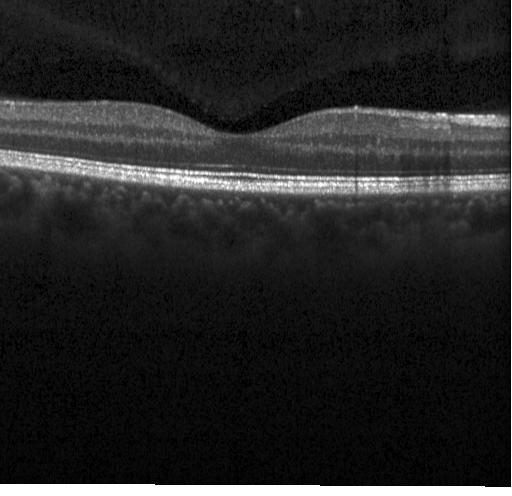 Instrument: Heidelberg Spectralis · spectral-domain optical coherence tomography · horizontal scan through the fovea · retinal OCT cross-section
This B-scan demonstrates neither choroidal neovascularization, diabetic macular edema, nor drusen.